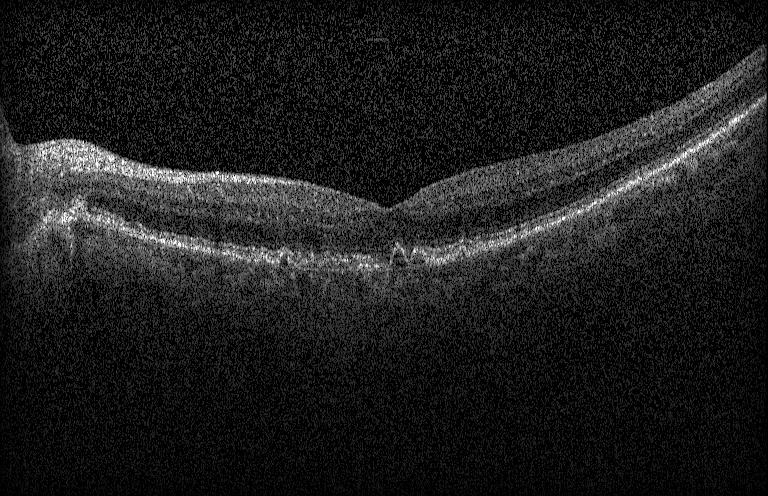

Fovea-centered; spectral-domain OCT; retinal OCT cross-section; instrument: Heidelberg Spectralis
Diagnosis: a choroidal neovascular membrane.